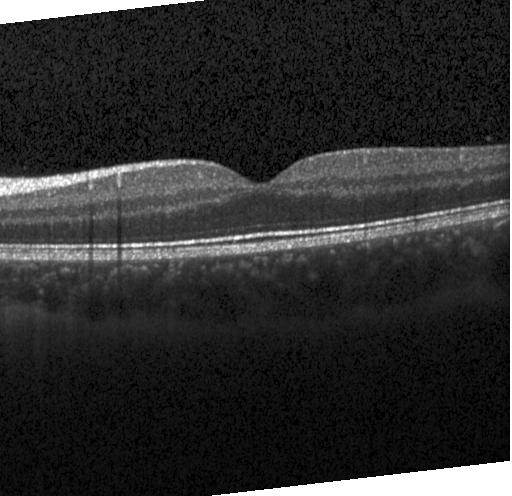 Heidelberg Spectralis; OCT line scan. Finding: no choroidal neovascularization, diabetic macular edema, or drusen.